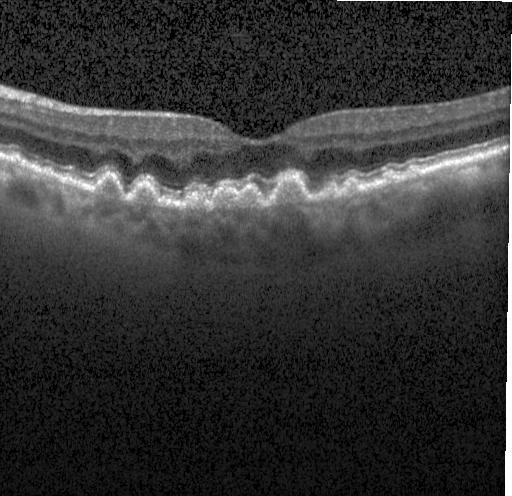 Instrument: Heidelberg Spectralis · OCT B-scan · through the macula · spectral-domain optical coherence tomography — Sub-RPE drusenoid deposits.